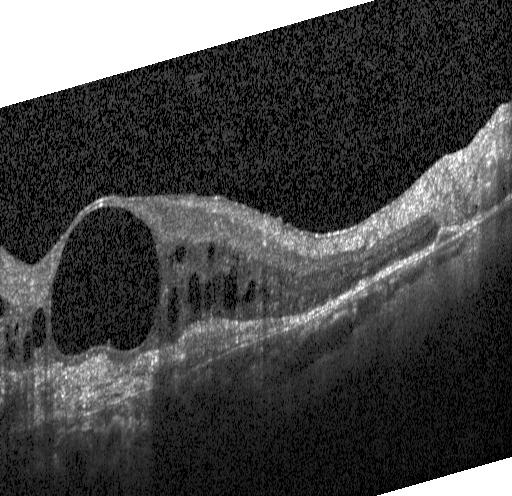 Assessment: a choroidal neovascular membrane.